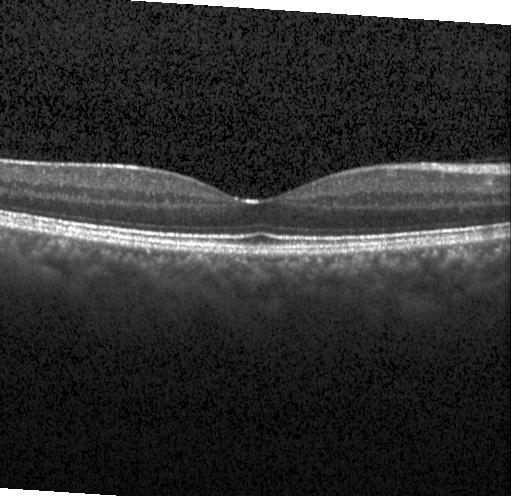 Macular scan · Heidelberg Spectralis · optical coherence tomography scan
Impression: no choroidal neovascularization, diabetic macular edema, or drusen.